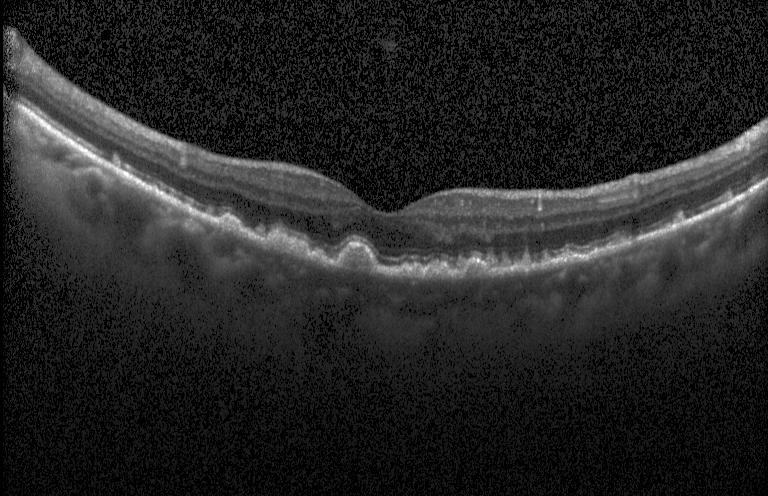
Macular scan; retinal OCT cross-section.
The scan shows sub-RPE drusenoid deposits.